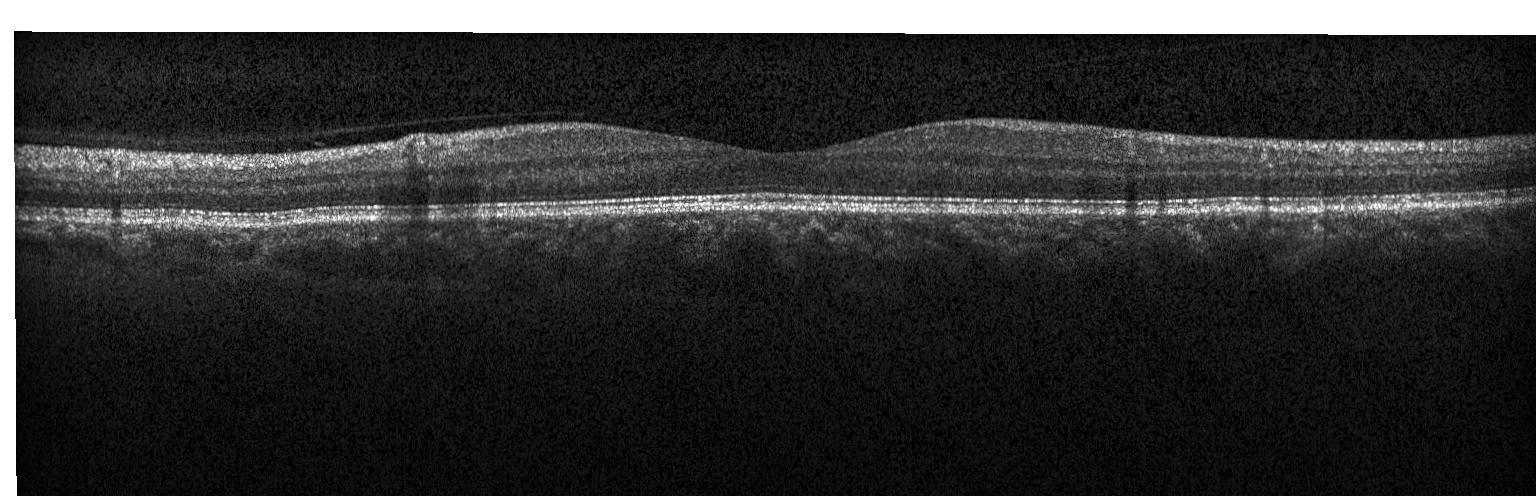
Finding: no choroidal neovascularization, diabetic macular edema, or drusen.